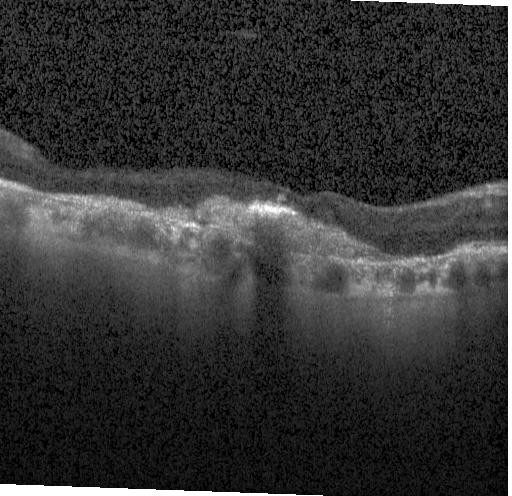 OCT finding: a choroidal neovascular membrane.